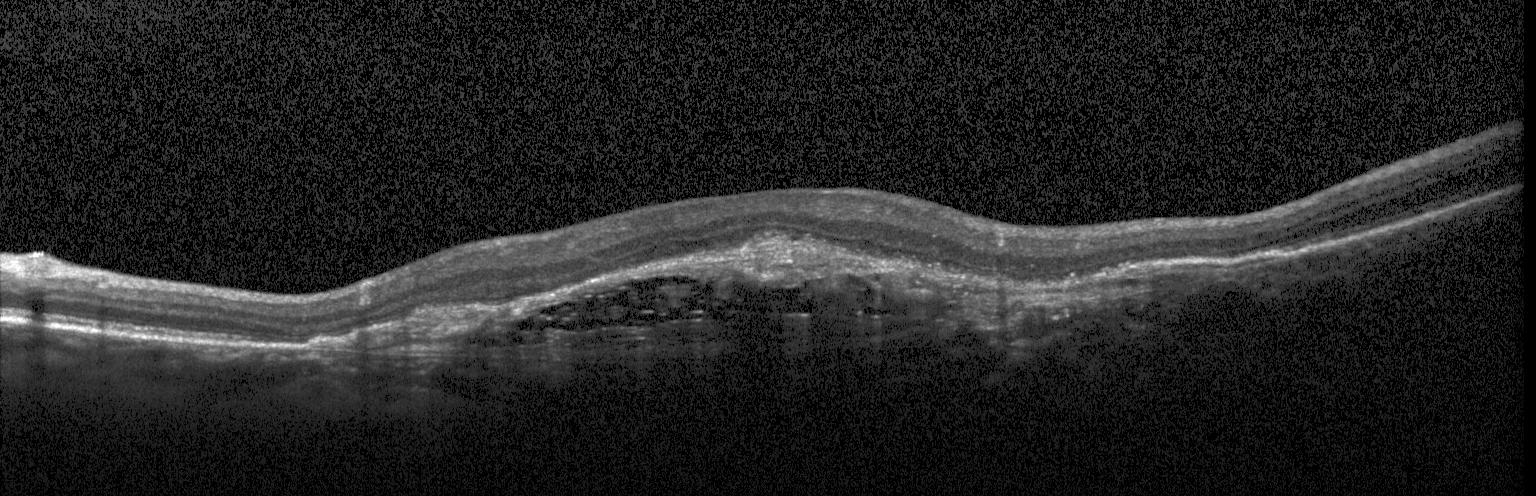

Macular OCT: CNV.